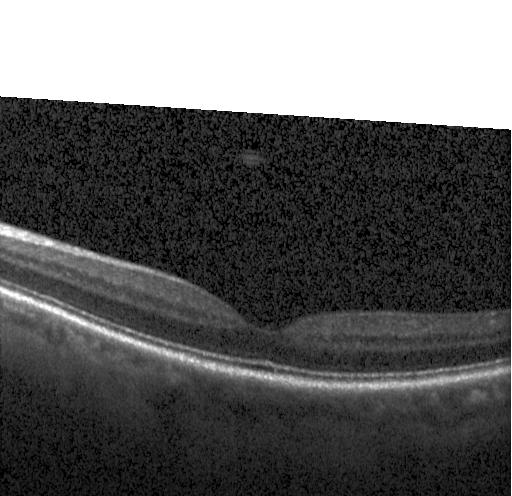

Impression: no CNV, no DME, and no drusen.